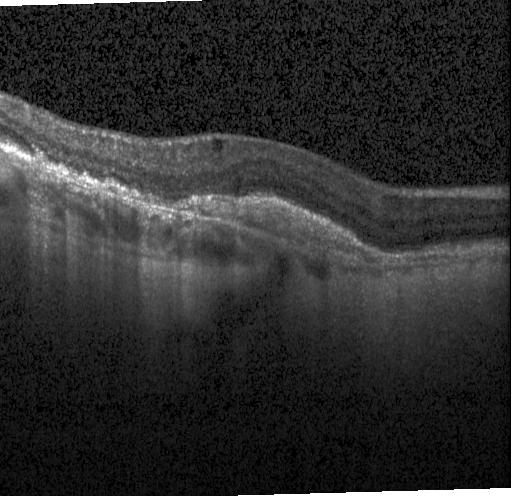 Instrument: Heidelberg Spectralis, spectral-domain optical coherence tomography, retinal OCT cross-section, horizontal scan through the fovea — A choroidal neovascular membrane.